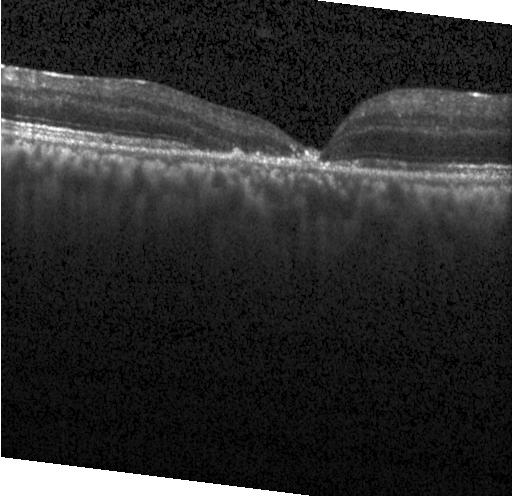 Diagnosis: no evidence of choroidal neovascularization, diabetic macular edema, or drusen.